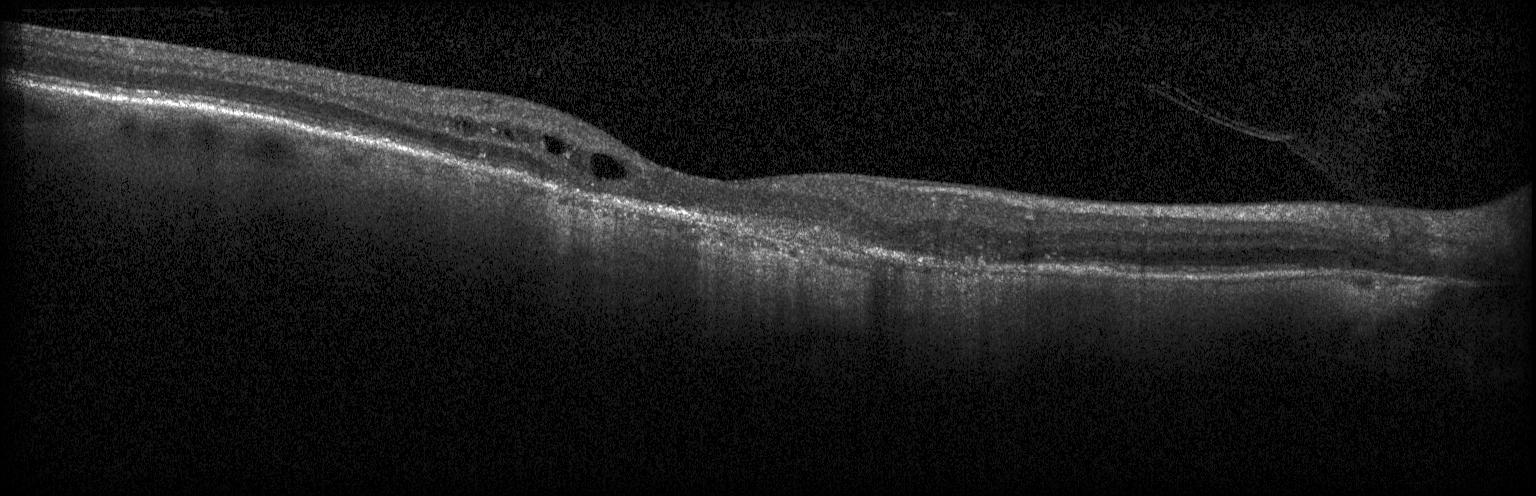
Assessment: choroidal neovascularization (CNV).